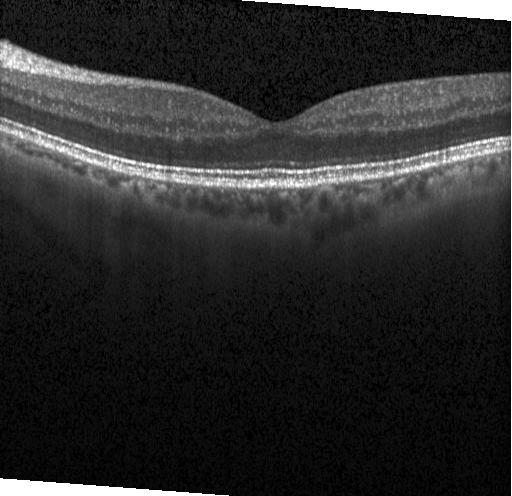
SD-OCT. Retinal OCT B-scan. Heidelberg Spectralis OCT system. This B-scan demonstrates neither choroidal neovascularization, diabetic macular edema, nor drusen.